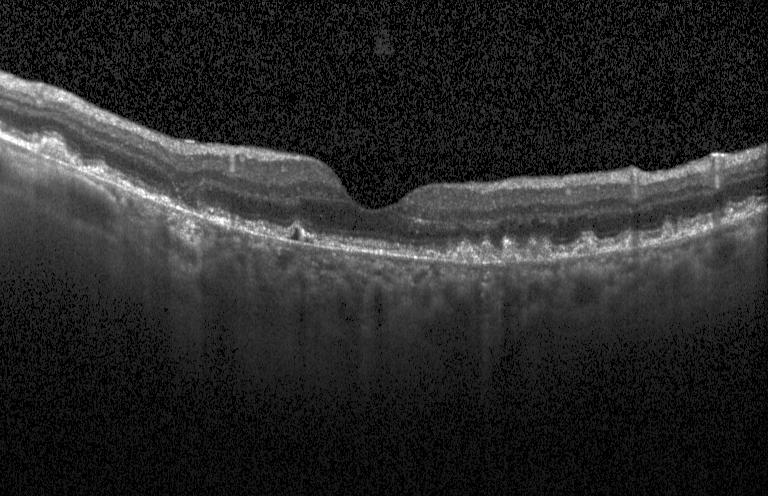

Finding: choroidal neovascularization.